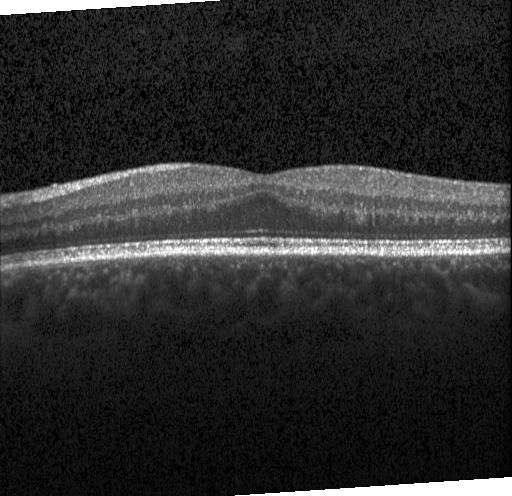

Diagnosis: no choroidal neovascularization, diabetic macular edema, or drusen.